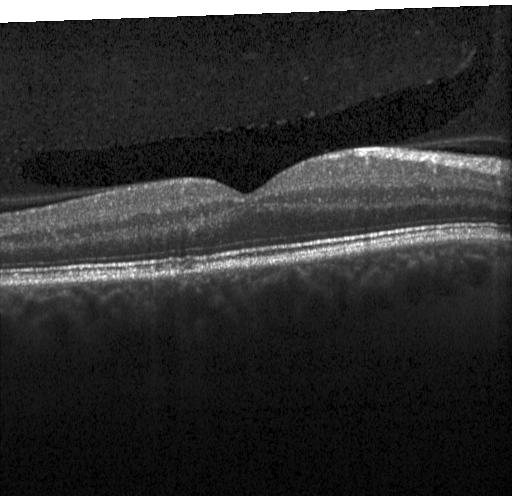

SD-OCT; retinal OCT B-scan.
Finding: no choroidal neovascularization, diabetic macular edema, or drusen.